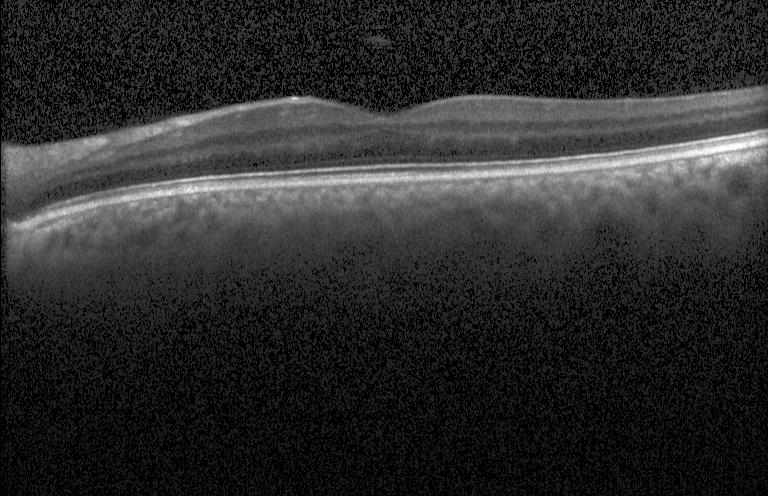

Diagnosis: no choroidal neovascularization, no diabetic macular edema, and no drusen.